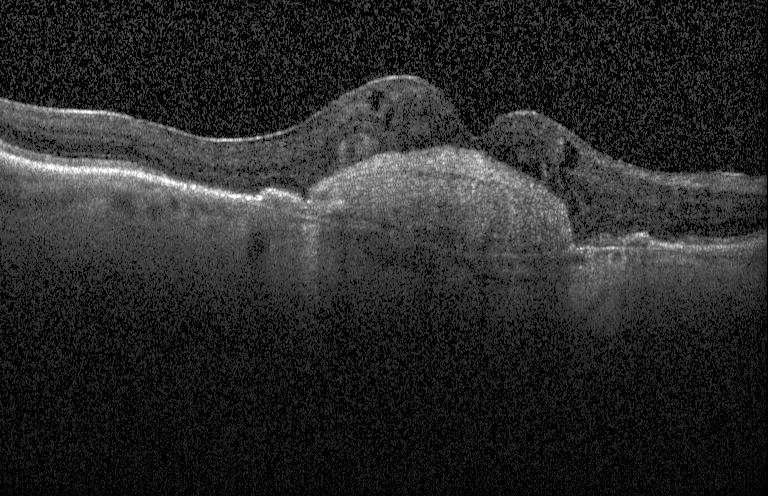
Impression: choroidal neovascularization.